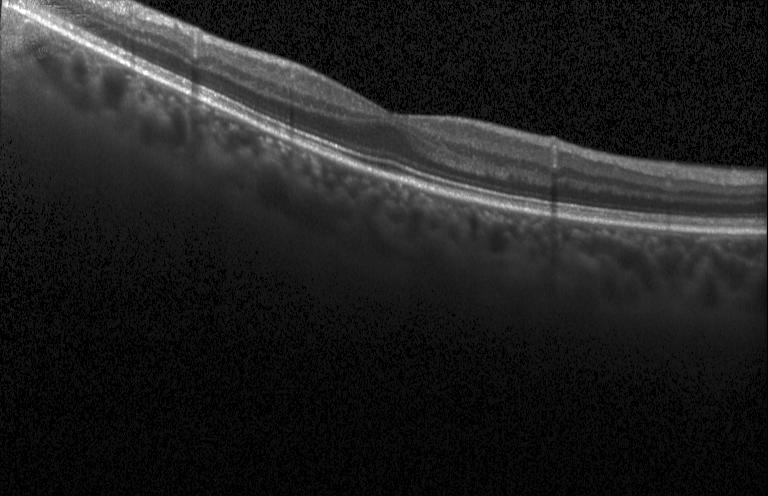 OCT B-scan, through the macula. Finding: no CNV, no DME, and no drusen.